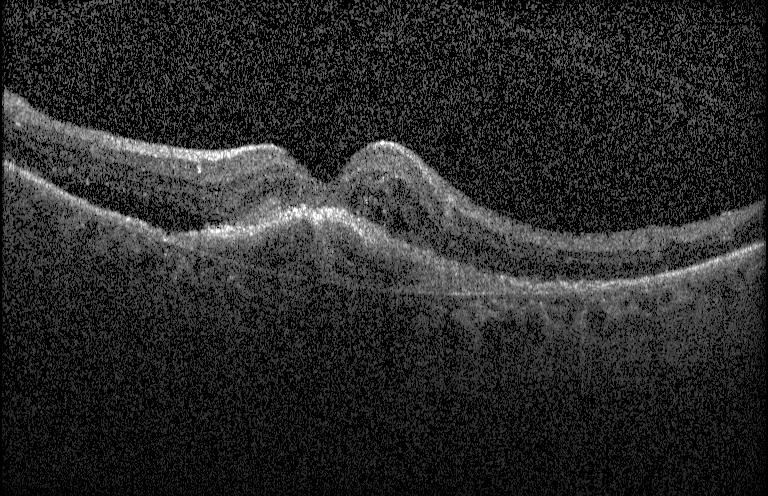

Spectral-domain optical coherence tomography · OCT line scan · Heidelberg Spectralis · horizontal scan through the fovea.
A choroidal neovascular membrane.